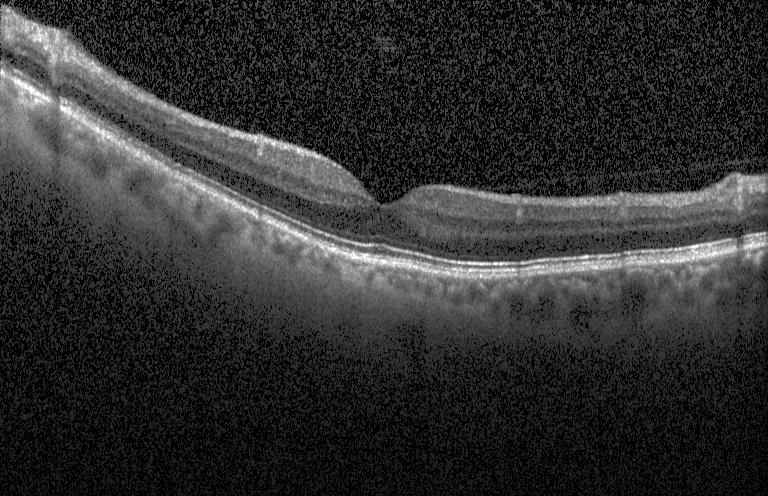 Instrument: Heidelberg Spectralis, spectral-domain optical coherence tomography, OCT B-scan, macular scan. The scan shows no CNV, DME, or drusen.